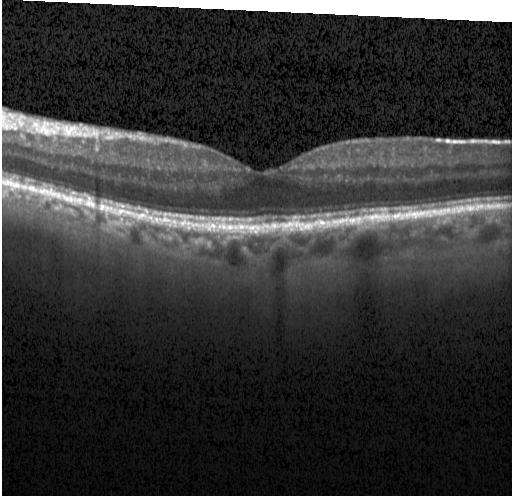

OCT scan showing no CNV, DME, or drusen.